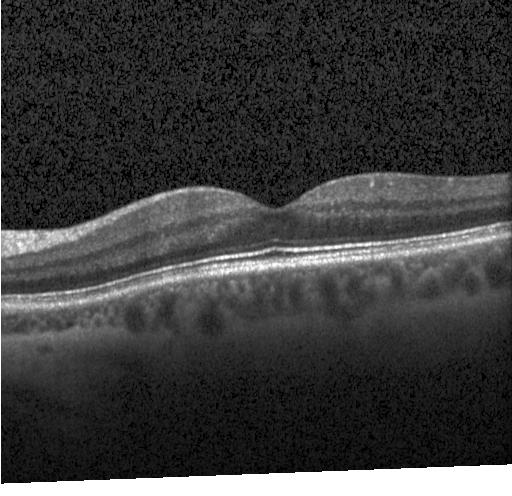
Heidelberg Spectralis; spectral-domain optical coherence tomography; OCT line scan. Impression: no choroidal neovascularization, diabetic macular edema, or drusen.